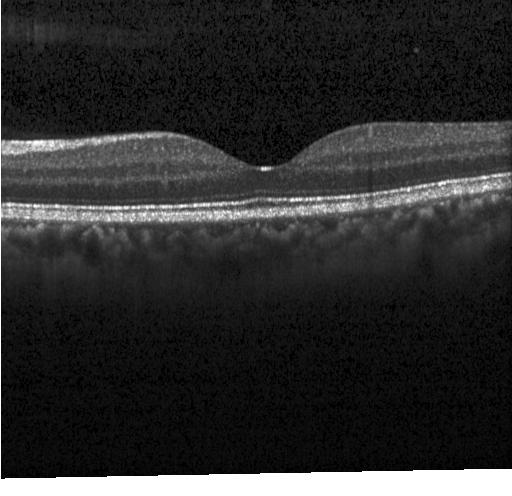 Dx: no choroidal neovascularization, no diabetic macular edema, and no drusen.